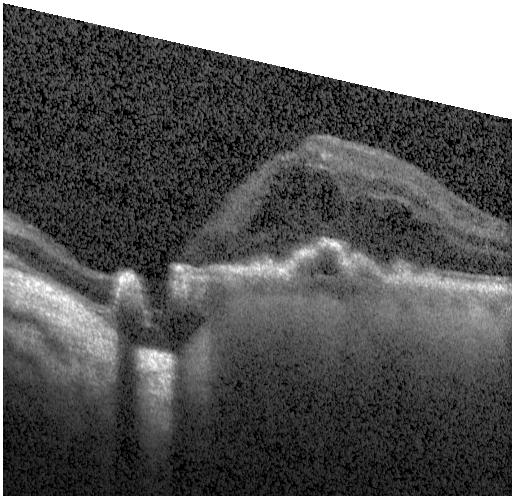 Acquired on a Heidelberg Spectralis. Spectral-domain optical coherence tomography. OCT B-scan — This B-scan demonstrates a choroidal neovascular membrane.